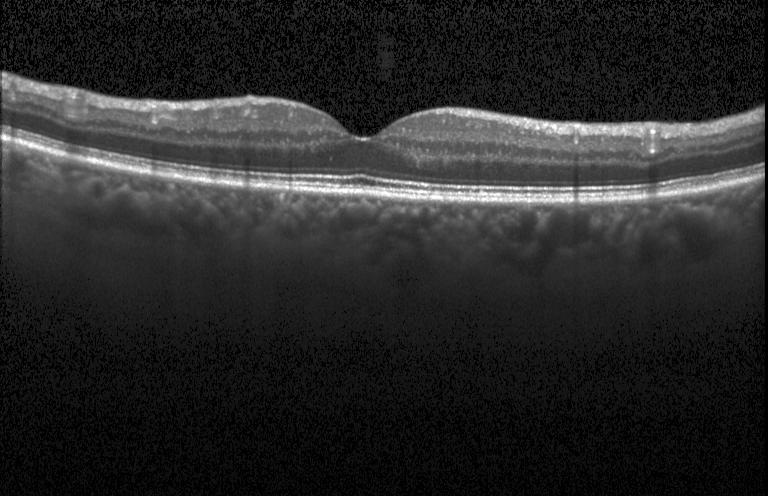
Centered on the fovea; OCT line scan — The scan shows neither CNV, DME, nor drusen.